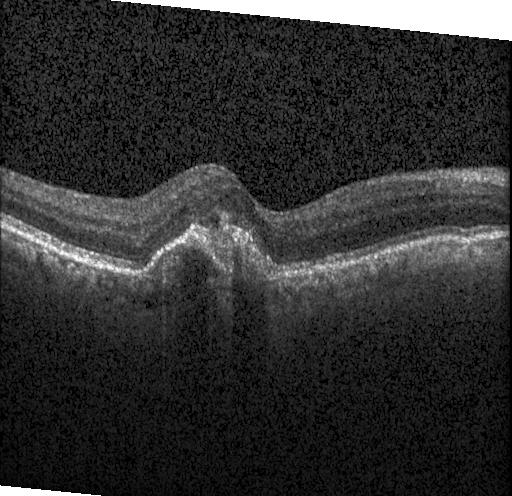

Dx: a choroidal neovascular membrane.